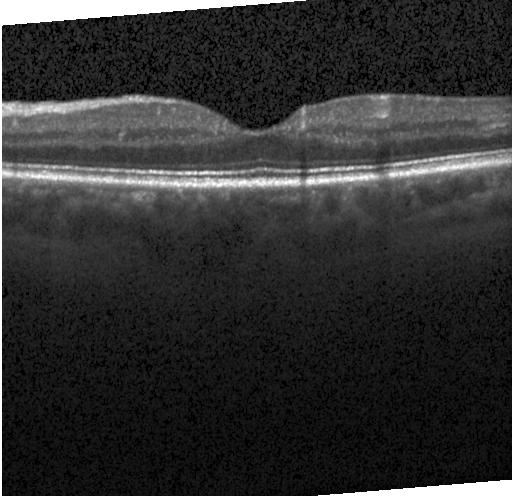
Impression: no CNV, DME, or drusen.